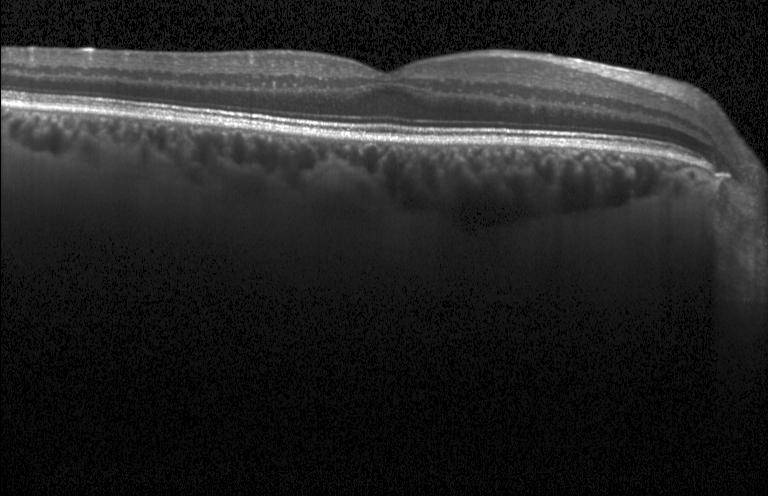

Assessment: no choroidal neovascularization, diabetic macular edema, or drusen.